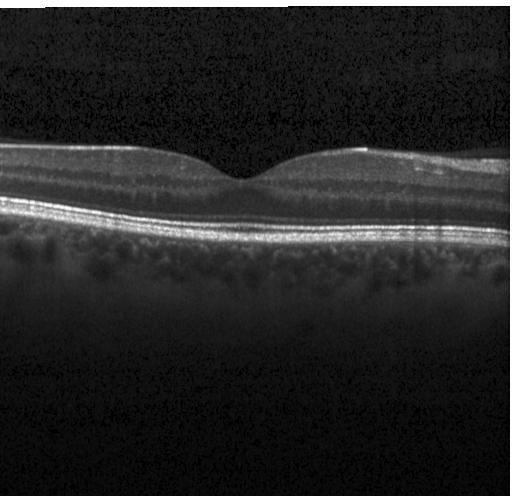 No choroidal neovascularization, diabetic macular edema, or drusen.